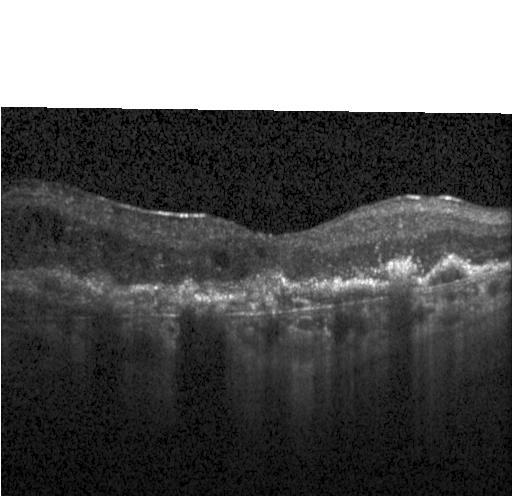 Heidelberg Spectralis OCT system; macular scan; OCT line scan. Finding: a choroidal neovascular membrane.